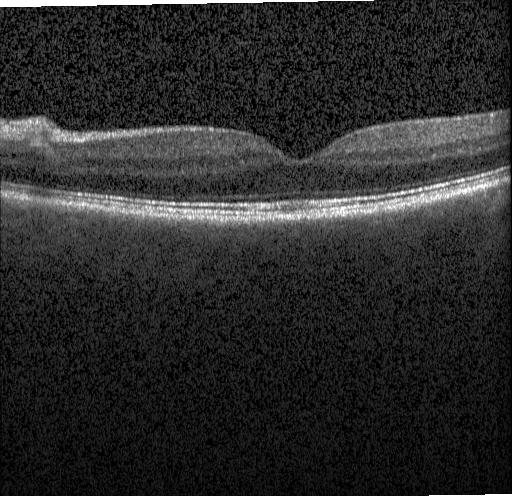

Diagnosis: no choroidal neovascularization, diabetic macular edema, or drusen.